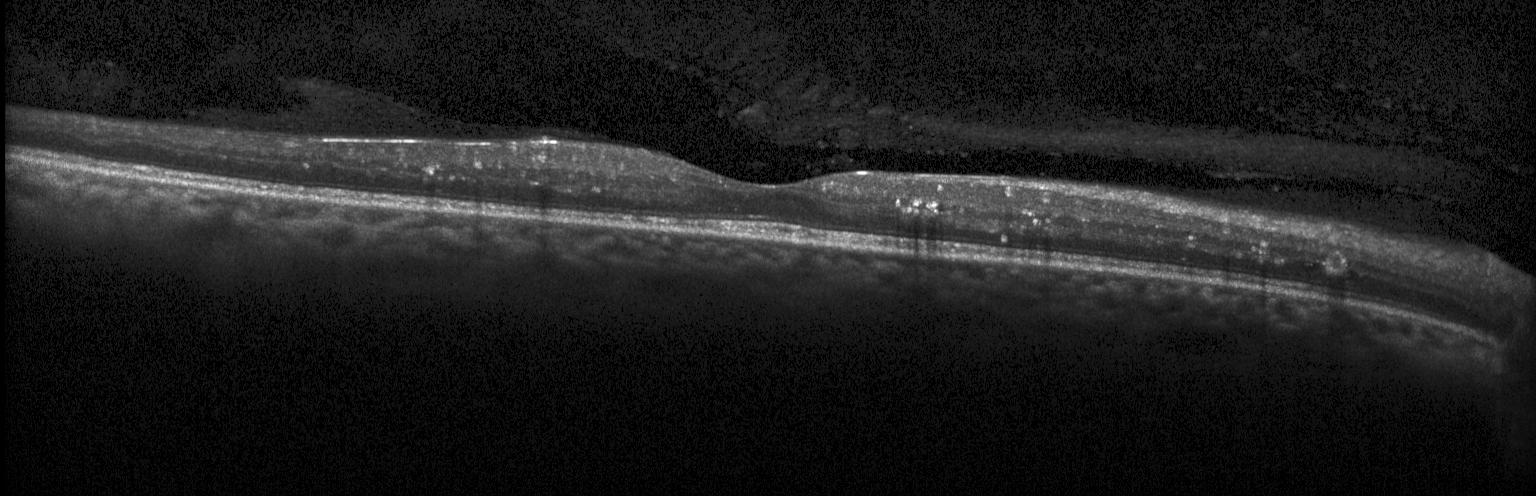 Spectral-domain OCT B-scan: diabetic macular edema.